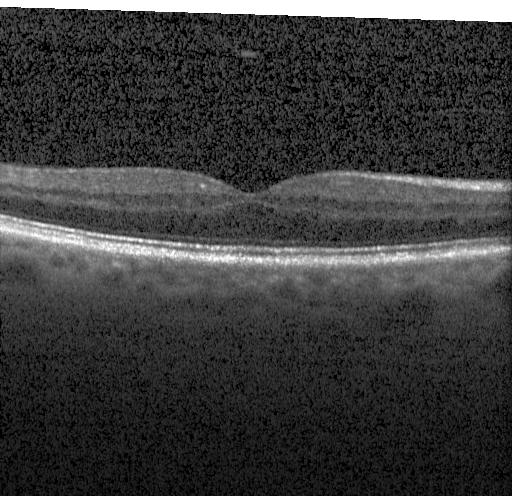
Retinal OCT B-scan, through the macula.
Impression: no CNV, DME, or drusen.